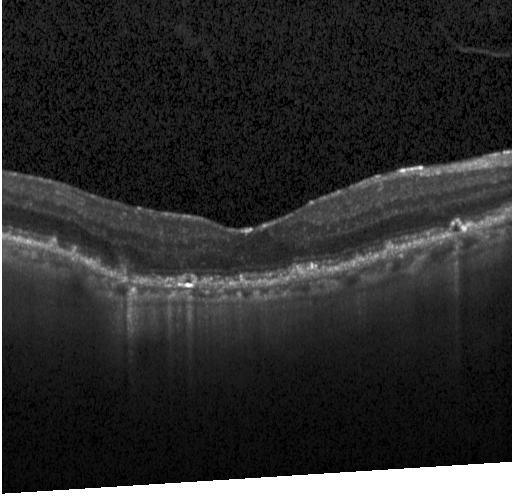 Retinal OCT B-scan · Heidelberg Spectralis · SD-OCT. OCT finding: a choroidal neovascular membrane.